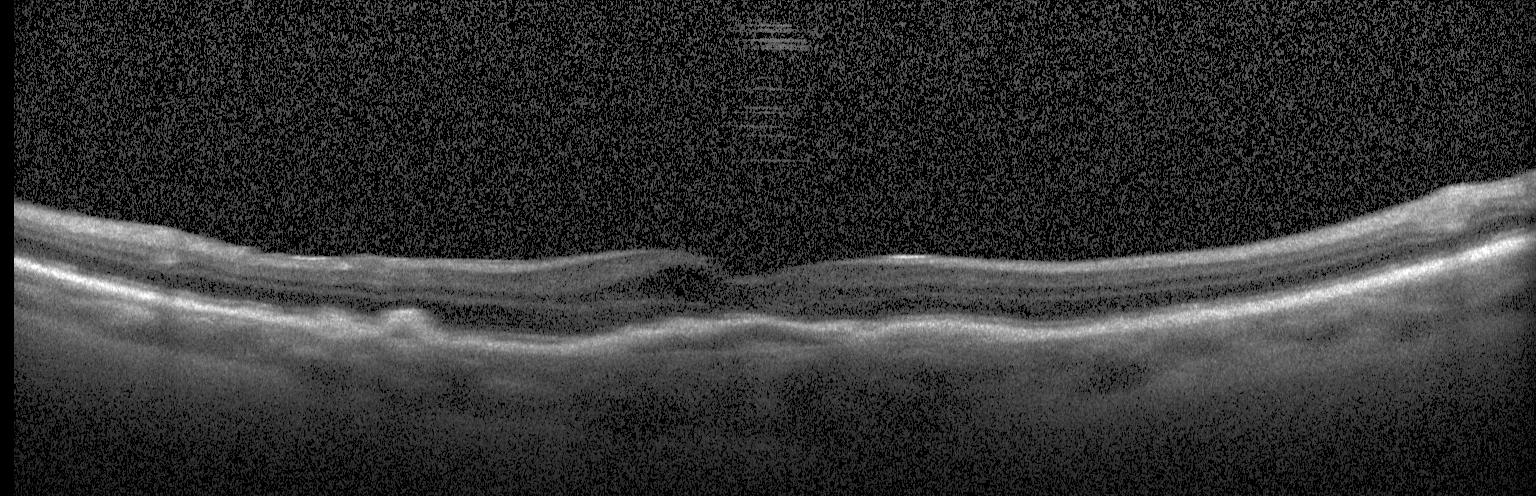 Fovea-centered, OCT line scan, Heidelberg Spectralis OCT system.
Impression: choroidal neovascularization.